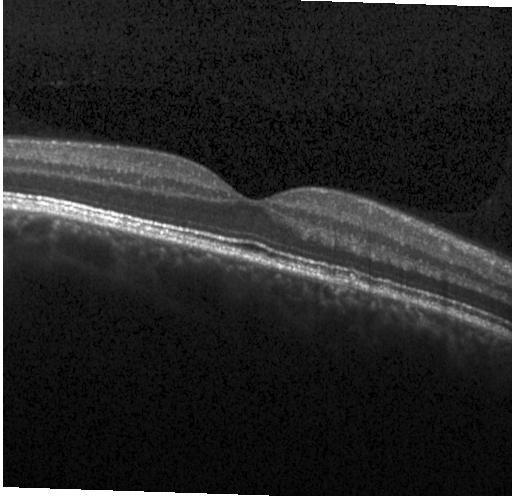

Optical coherence tomography B-scan. Finding: neither choroidal neovascularization, diabetic macular edema, nor drusen.